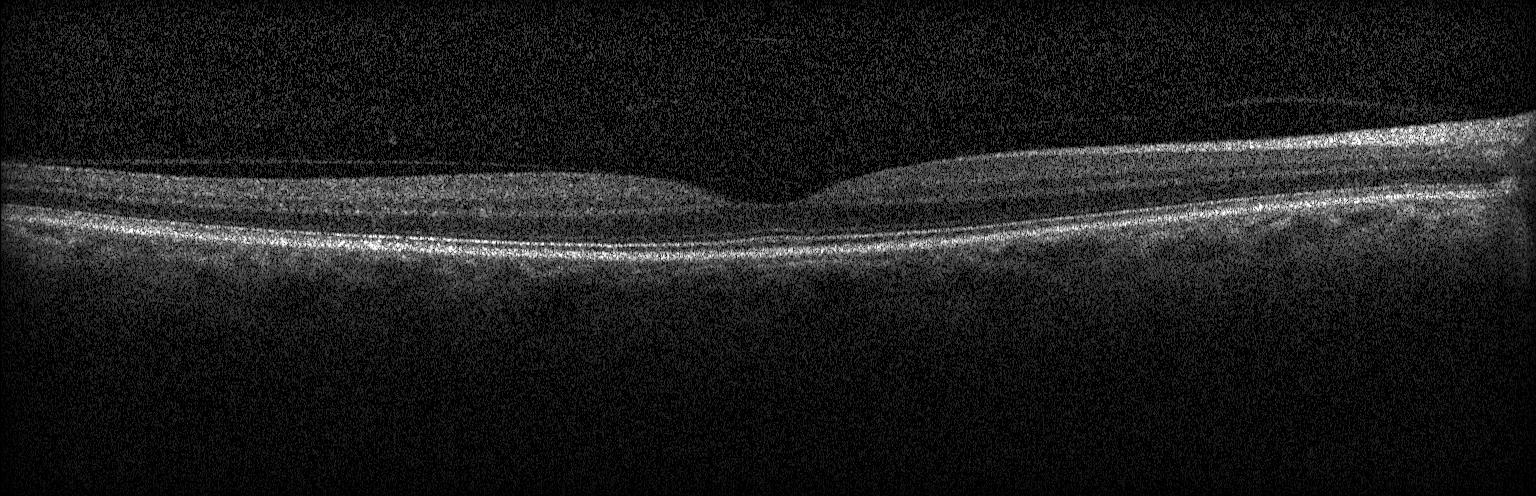 OCT B-scan. Impression: no choroidal neovascularization, diabetic macular edema, or drusen.